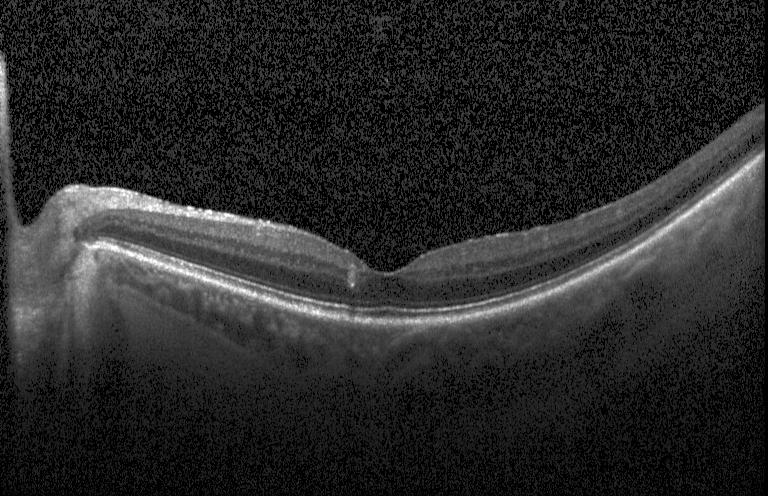
Macular OCT demonstrating neither choroidal neovascularization, diabetic macular edema, nor drusen.